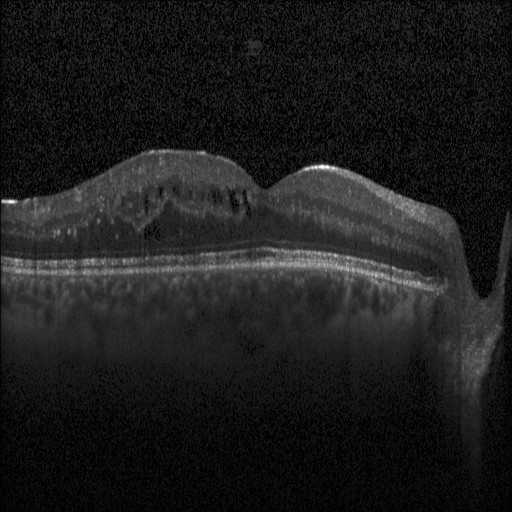 Retinal OCT B-scan; acquired on a Heidelberg Spectralis; centered on the fovea. Finding: DME.